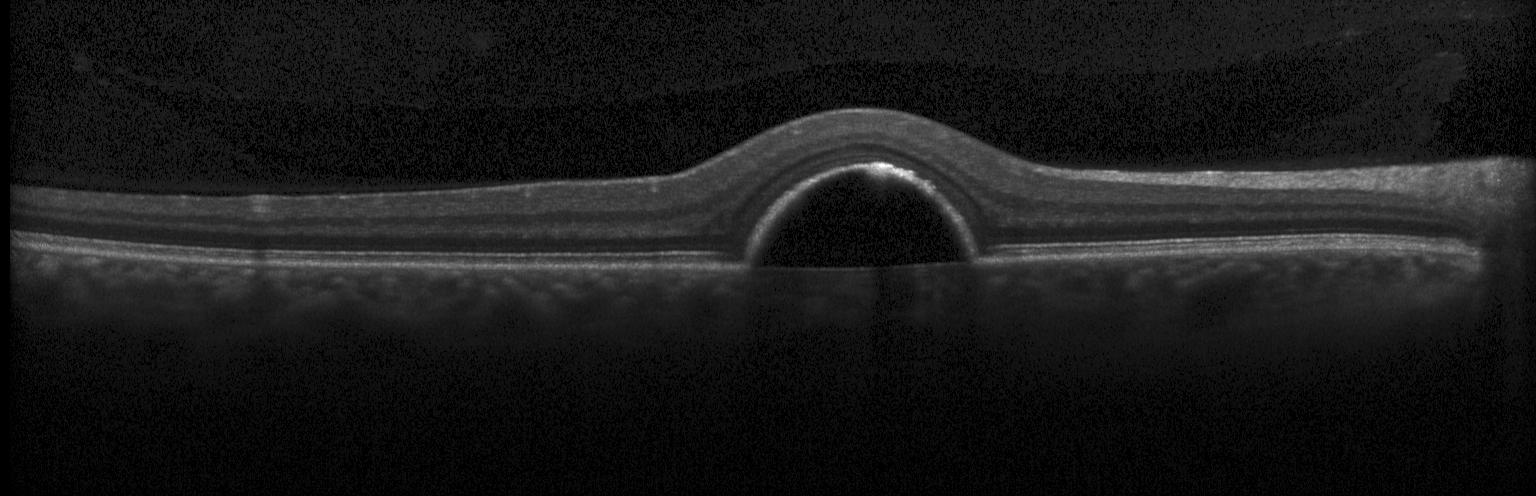
OCT B-scan · through the macula · spectral-domain OCT — Assessment: CNV.